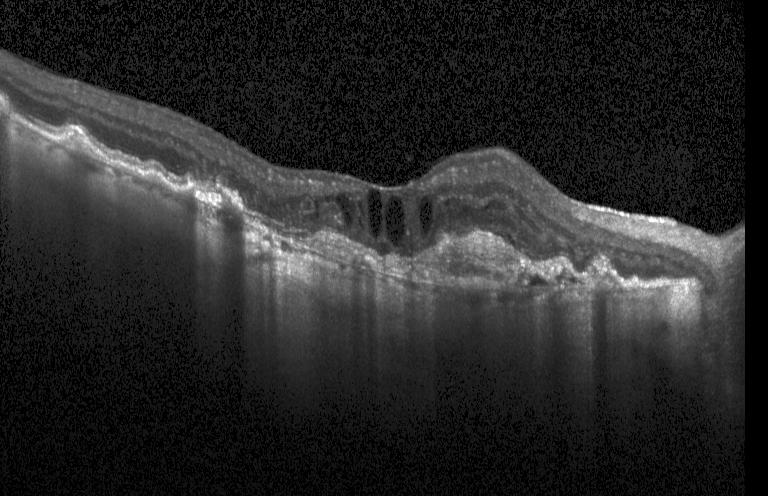 Finding: a choroidal neovascular membrane.